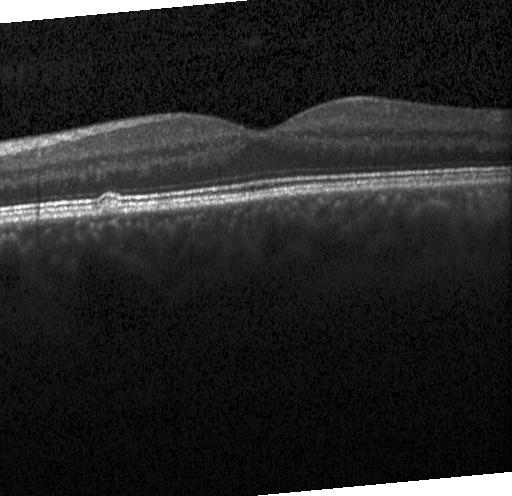
Finding: multiple drusen.